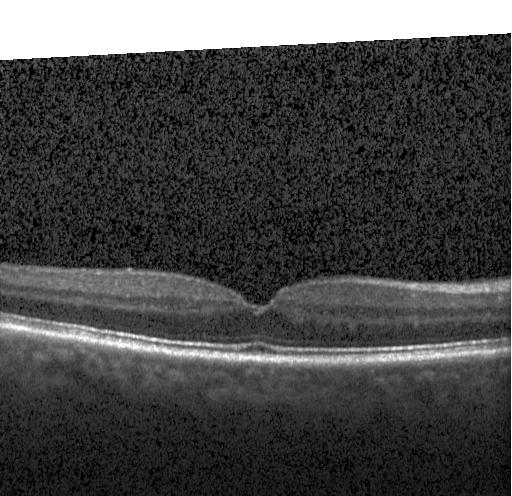 OCT line scan.
Finding: no CNV, DME, or drusen.